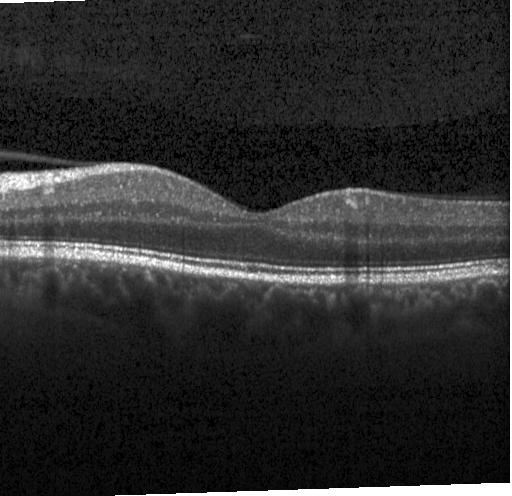

Retinal OCT B-scan — Diagnosis: no CNV, DME, or drusen.